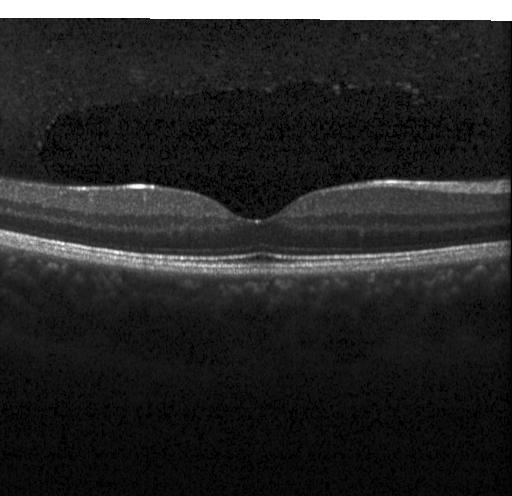
Retinal OCT B-scan
Impression: no evidence of CNV, DME, or drusen.